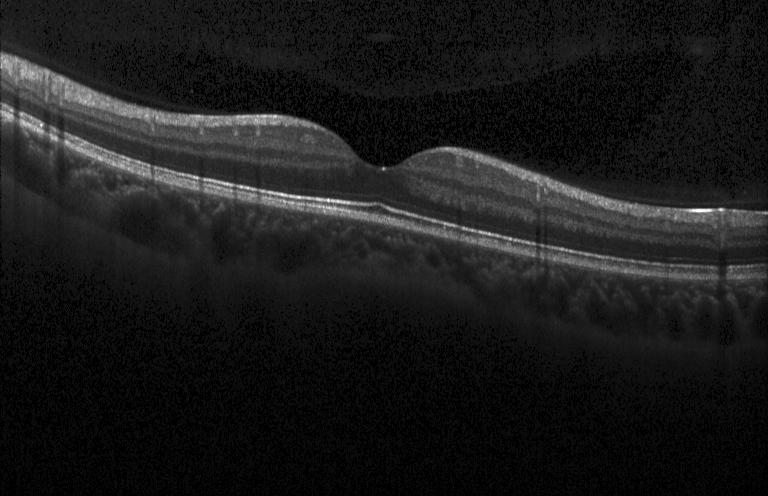 Macular OCT demonstrating neither choroidal neovascularization, diabetic macular edema, nor drusen.